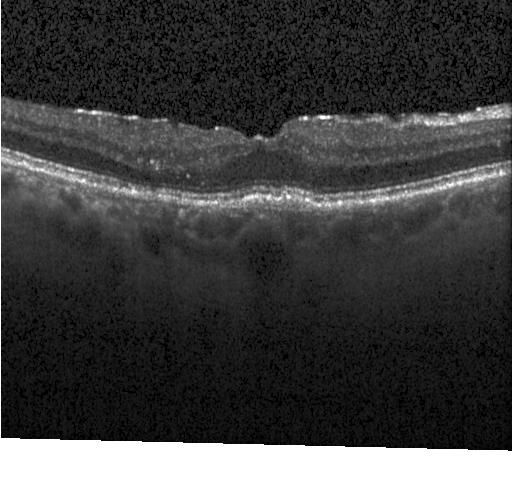

Spectral-domain optical coherence tomography · OCT line scan.
This B-scan demonstrates CNV.